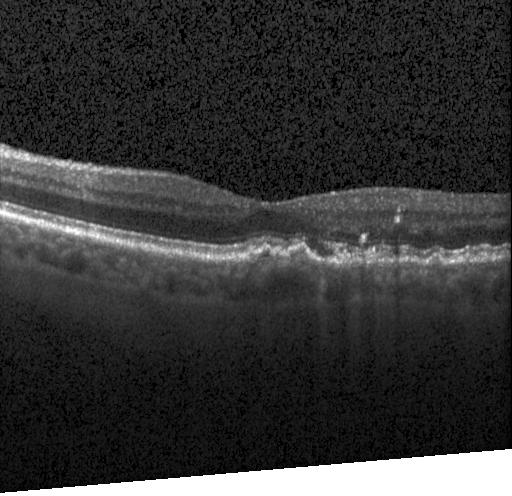

Instrument: Heidelberg Spectralis; optical coherence tomography B-scan
The scan shows sub-RPE drusenoid deposits.